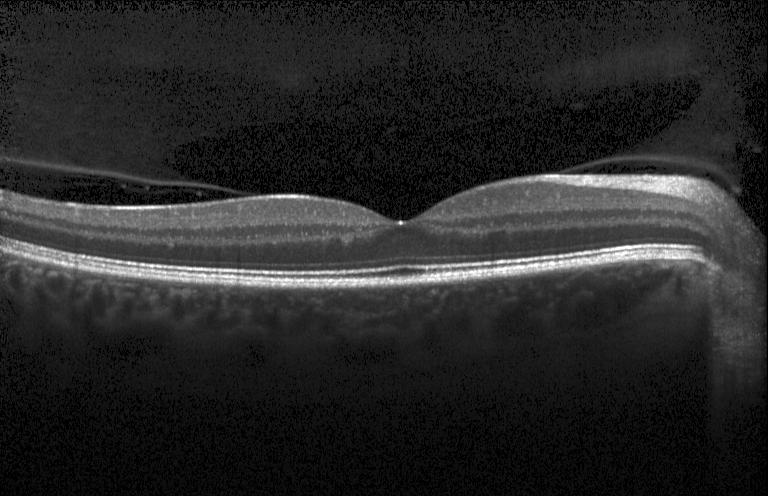

Through the macula. OCT line scan. Heidelberg Spectralis OCT system.
This B-scan demonstrates neither choroidal neovascularization, diabetic macular edema, nor drusen.